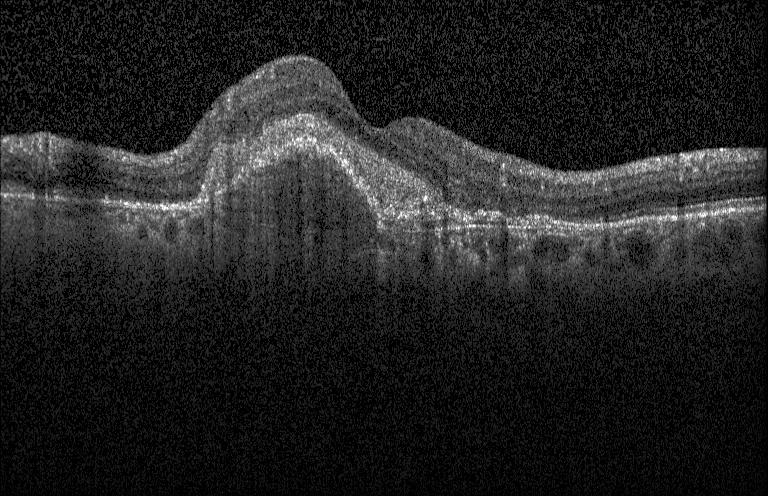
The scan shows choroidal neovascularization.